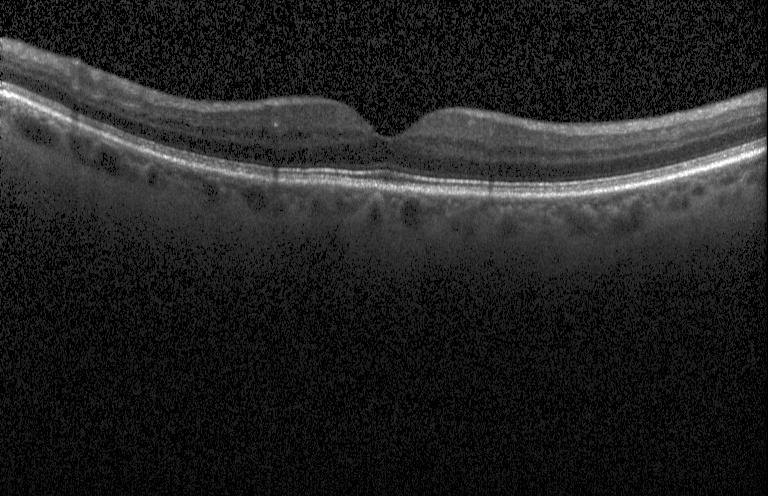

Spectral-domain optical coherence tomography · fovea-centered · optical coherence tomography scan — OCT finding: no evidence of choroidal neovascularization, diabetic macular edema, or drusen.